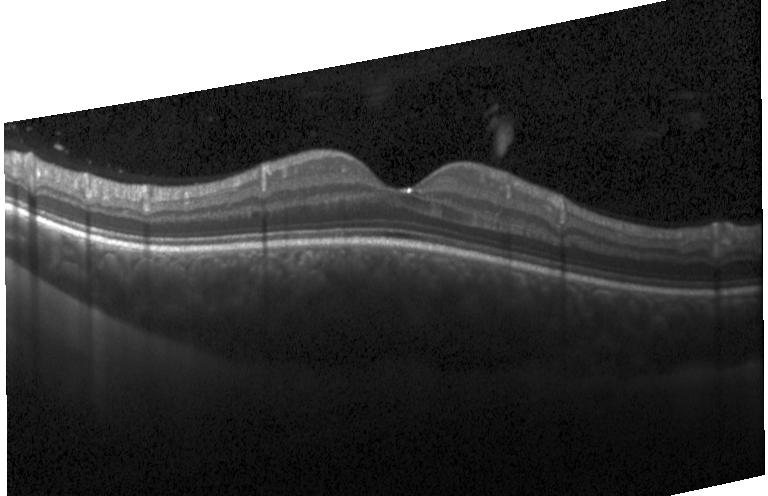

Impression: no CNV, no DME, and no drusen.